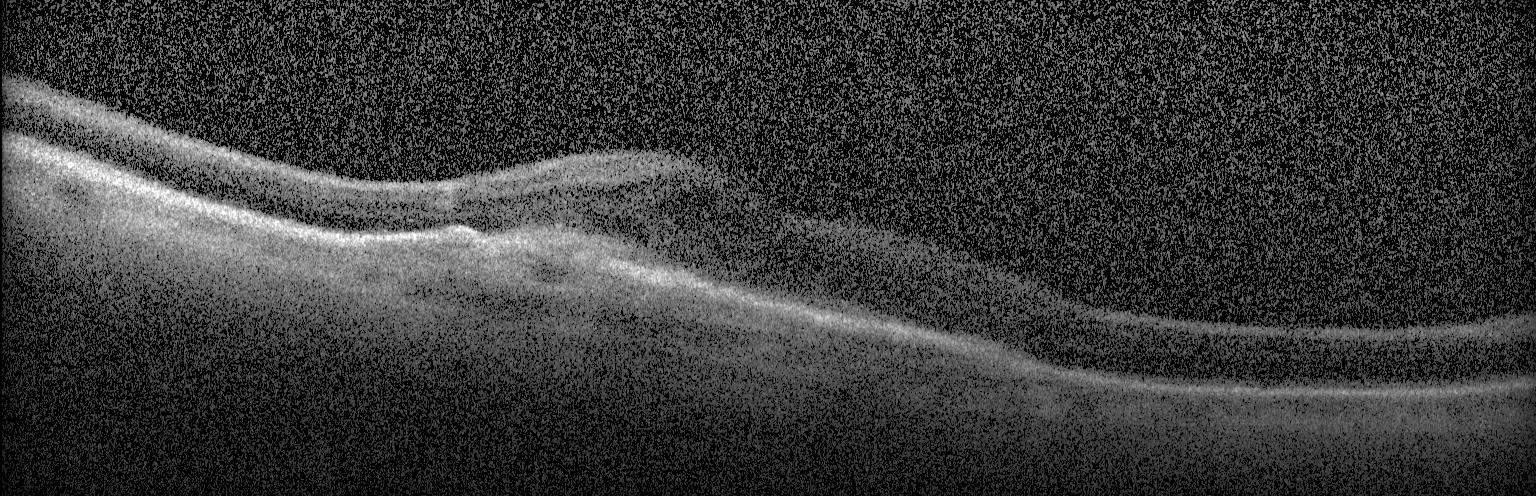 The scan shows choroidal neovascularization.